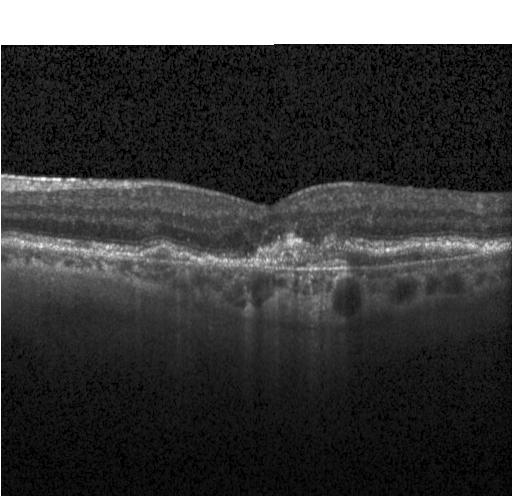 Optical coherence tomography B-scan. Spectral-domain OCT. Heidelberg Spectralis
A choroidal neovascular membrane.